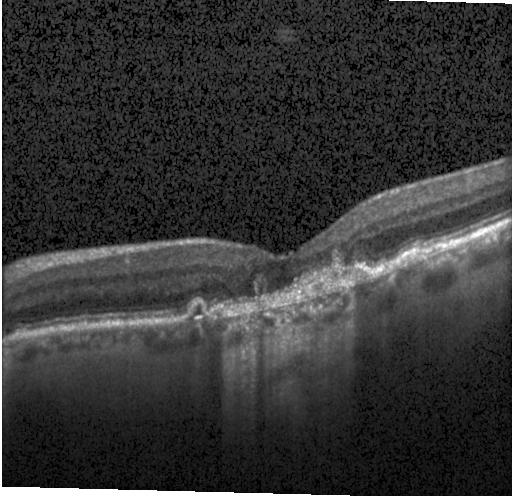 Retinal OCT B-scan; horizontal scan through the fovea; instrument: Heidelberg Spectralis; SD-OCT.
Dx: a choroidal neovascular membrane.